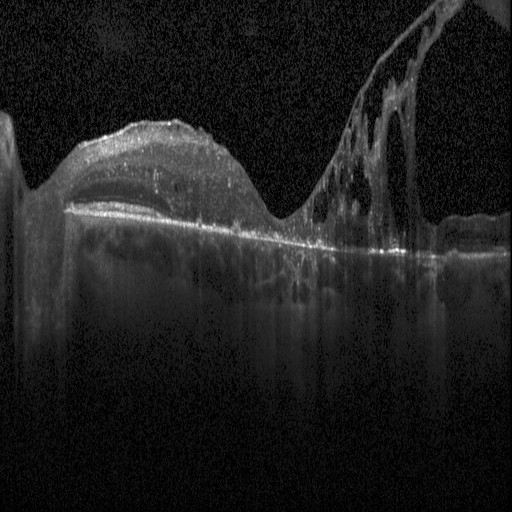 Horizontal scan through the fovea · optical coherence tomography B-scan.
Diagnosis: DME.